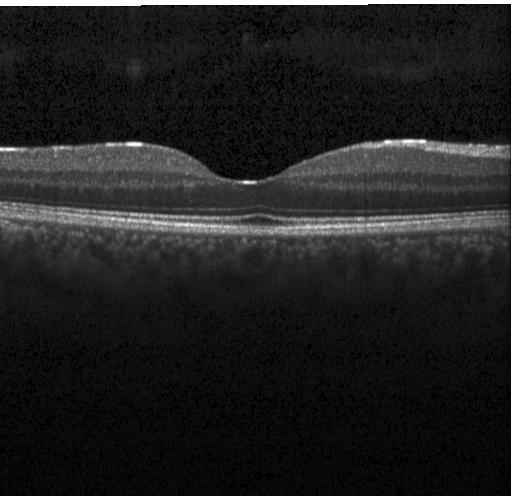
Spectral-domain optical coherence tomography · macular scan · acquired on a Heidelberg Spectralis · optical coherence tomography B-scan — Neither choroidal neovascularization, diabetic macular edema, nor drusen.